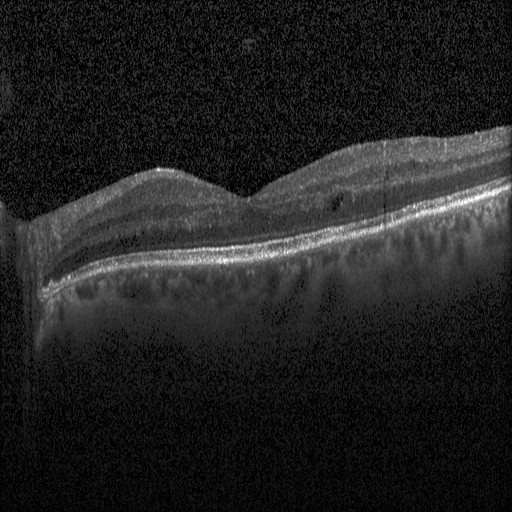

Spectral-domain optical coherence tomography · retinal OCT B-scan.
Diabetic macular edema (DME).